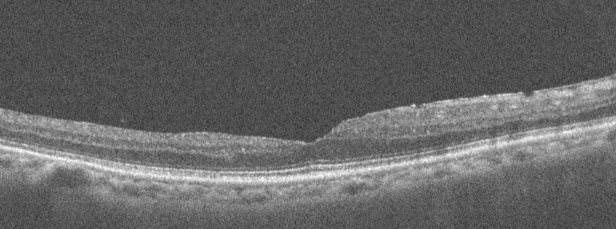 OCT line scan · Optovue Avanti RTVue XR · macular scan — Dx: epiretinal membrane.